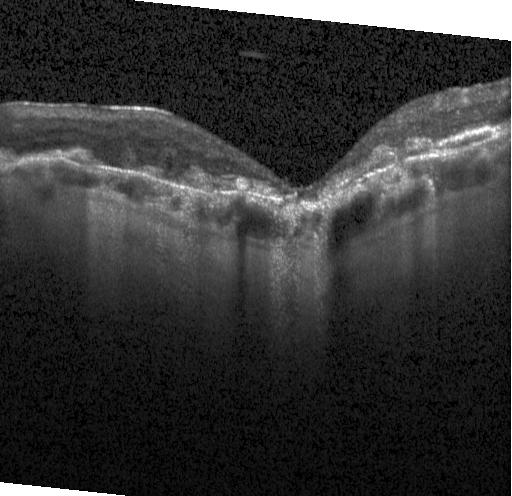 Heidelberg Spectralis OCT system · centered on the fovea · OCT line scan — Finding: CNV.